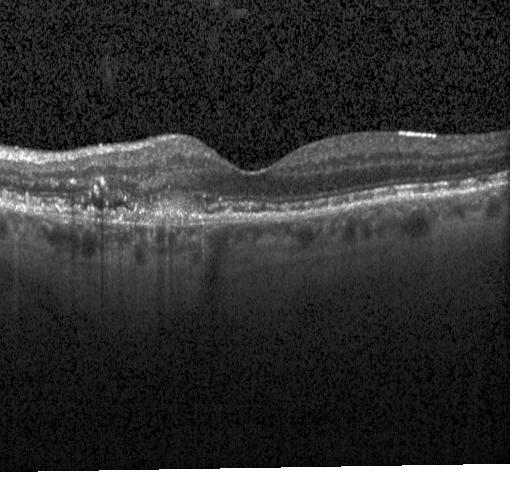
OCT B-scan; SD-OCT. Diagnosis: CNV.